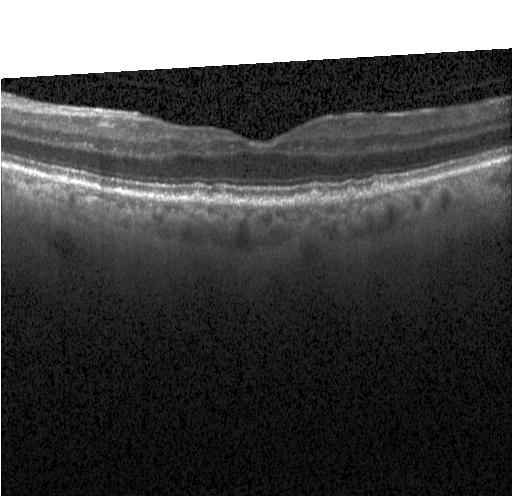

Finding: sub-RPE drusenoid deposits.